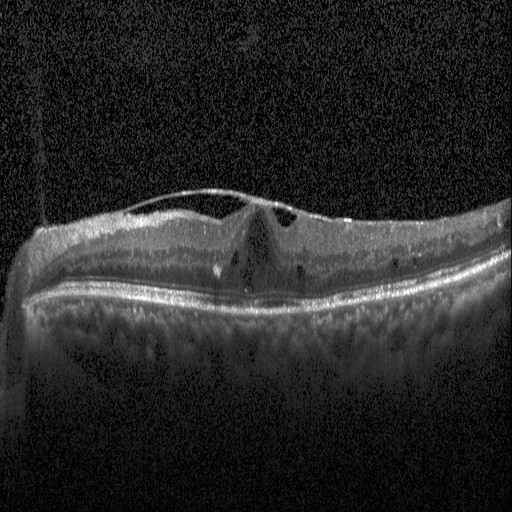 Retinal OCT B-scan · through the macula · spectral-domain OCT. Diagnosis: DME.